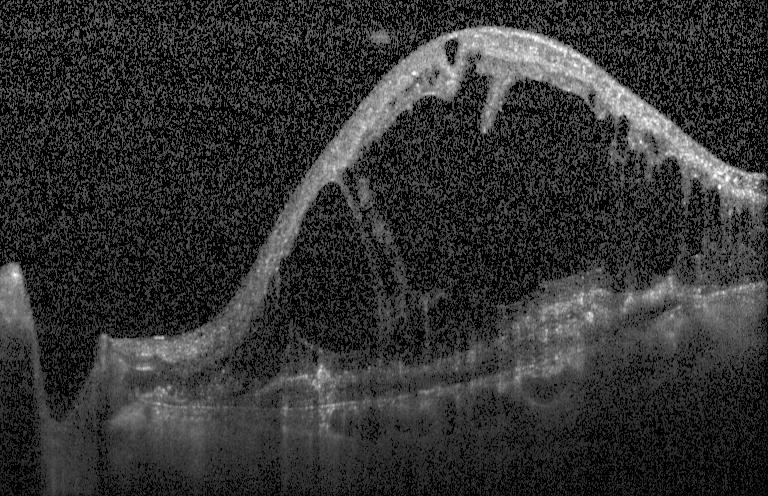 Optical coherence tomography B-scan. Heidelberg Spectralis. Spectral-domain optical coherence tomography — The scan shows CNV.